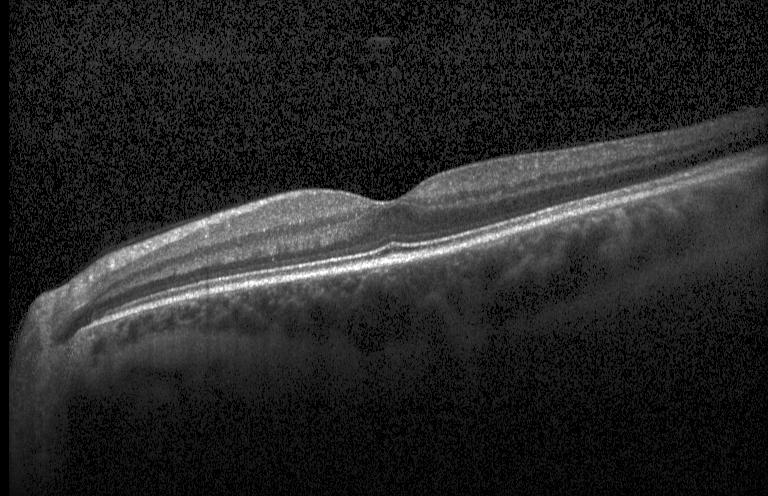 The scan shows neither choroidal neovascularization, diabetic macular edema, nor drusen.